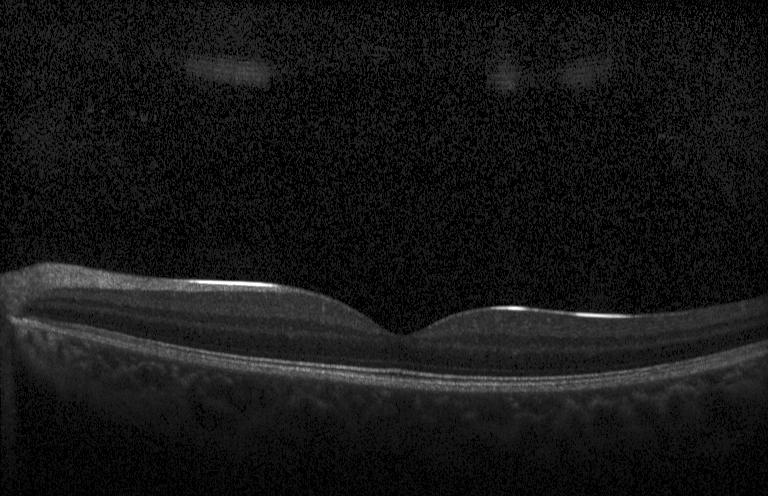
OCT B-scan
The scan shows no evidence of choroidal neovascularization, diabetic macular edema, or drusen.